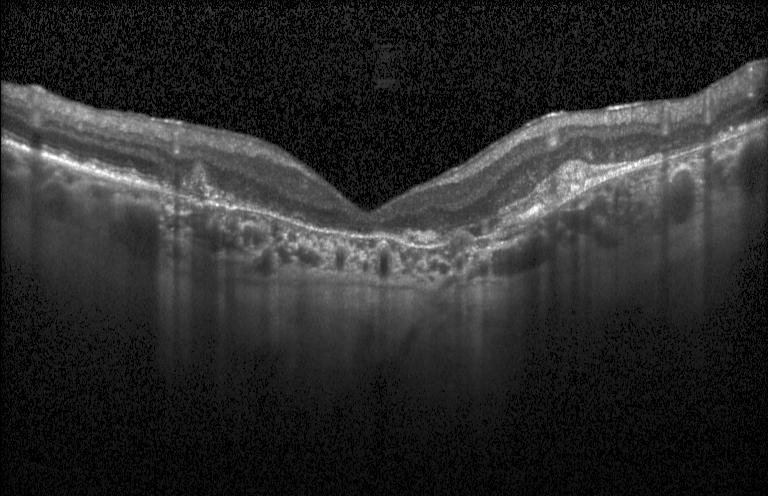

Spectral-domain OCT · optical coherence tomography B-scan
A choroidal neovascular membrane.